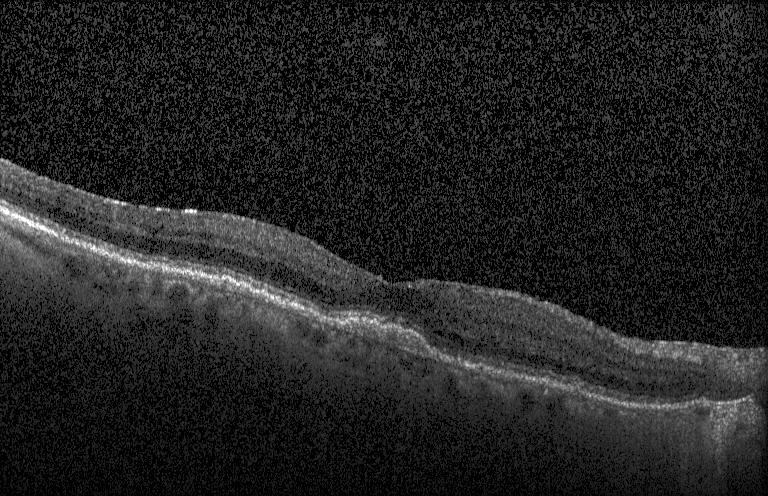 This B-scan demonstrates a choroidal neovascular membrane.